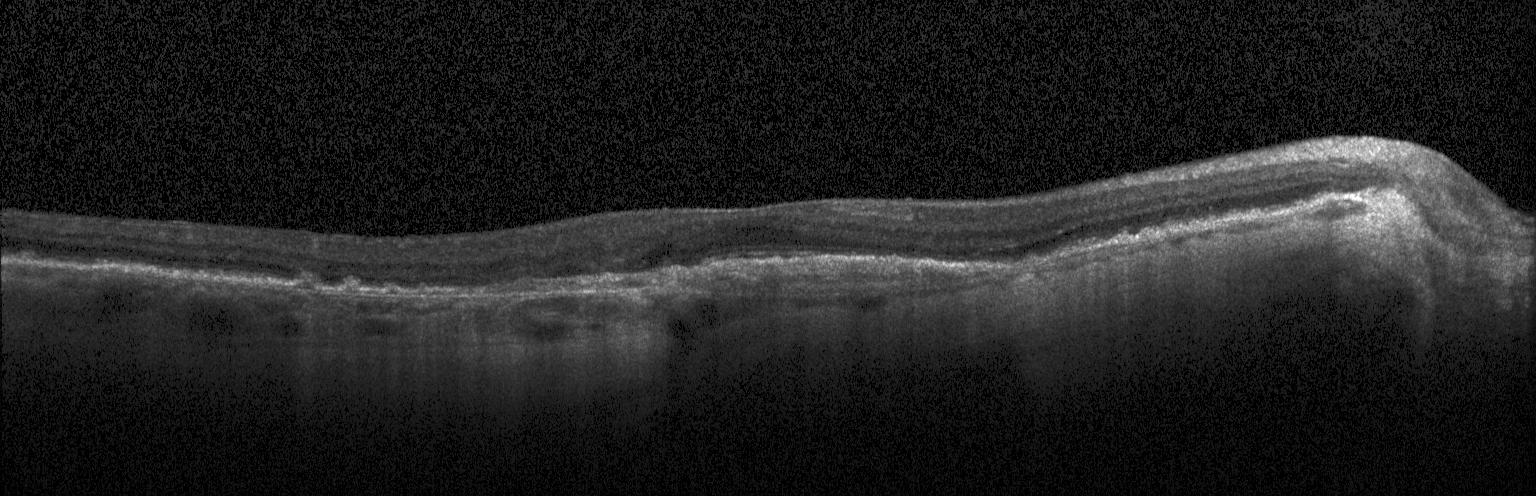

Spectral-domain optical coherence tomography. Acquired on a Heidelberg Spectralis. Retinal OCT B-scan. Macular scan
Finding: choroidal neovascularization.